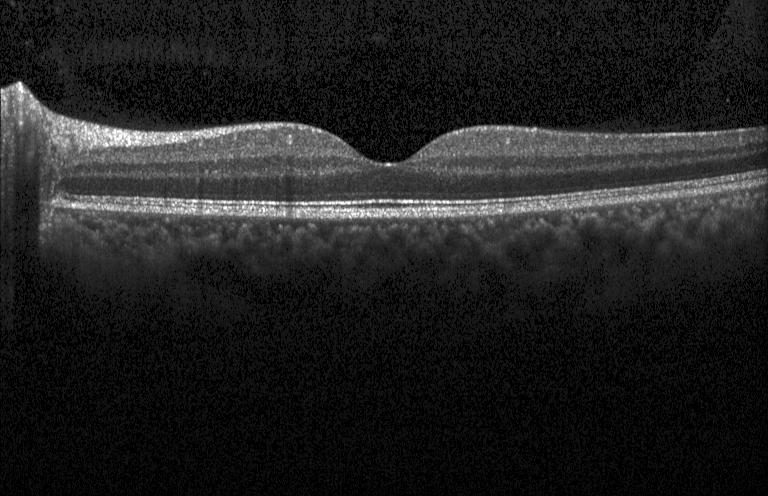

OCT line scan · through the macula. Finding: no choroidal neovascularization, diabetic macular edema, or drusen.